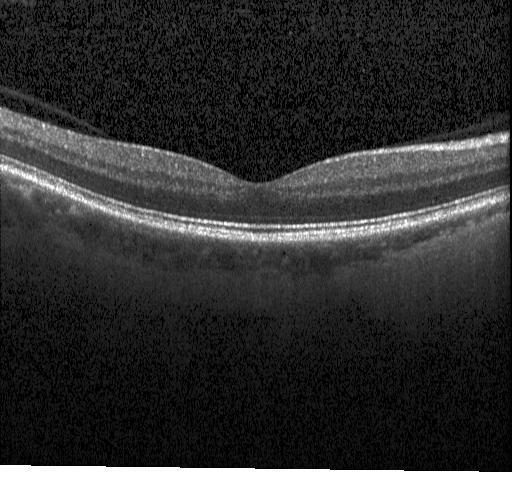 Optical coherence tomography scan. Heidelberg Spectralis OCT system. Through the macula.
Macular OCT: no choroidal neovascularization, no diabetic macular edema, and no drusen.